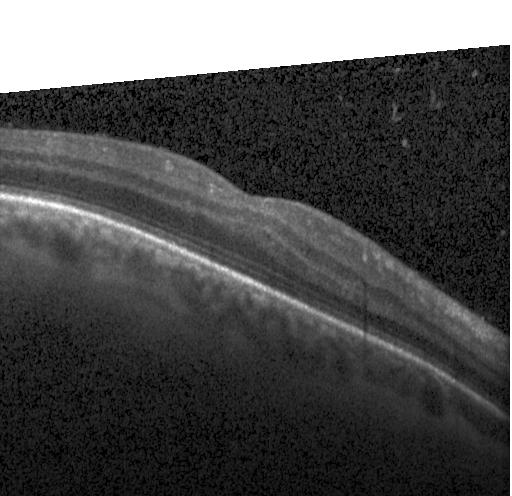

No choroidal neovascularization, diabetic macular edema, or drusen.